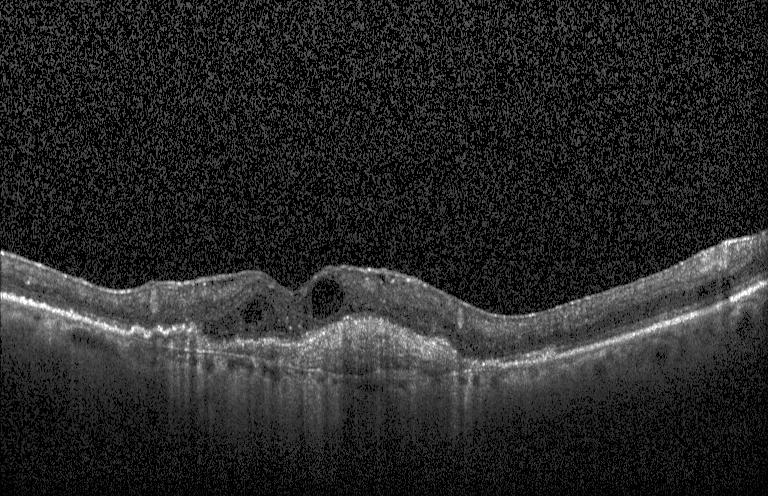
The scan shows a choroidal neovascular membrane.